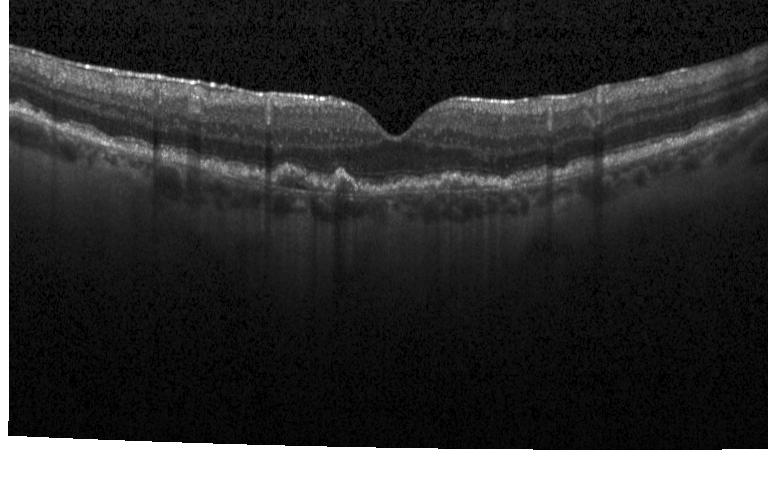 Retinal OCT B-scan; SD-OCT; fovea-centered; acquired on a Heidelberg Spectralis — Assessment: drusen.